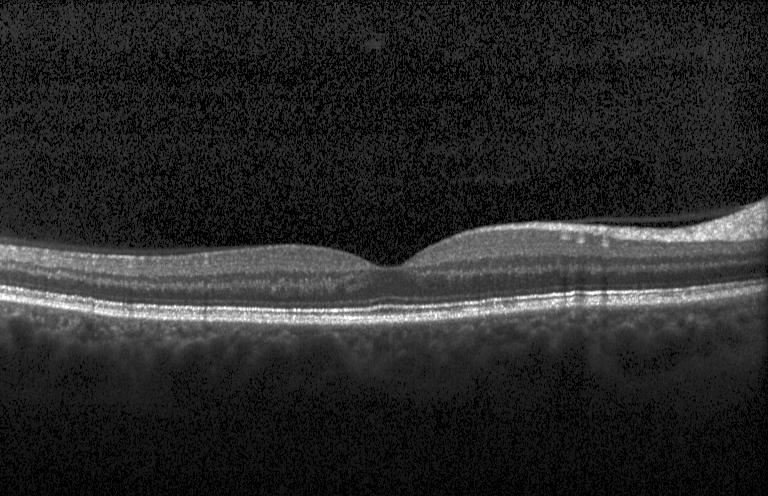 This B-scan demonstrates neither CNV, DME, nor drusen.